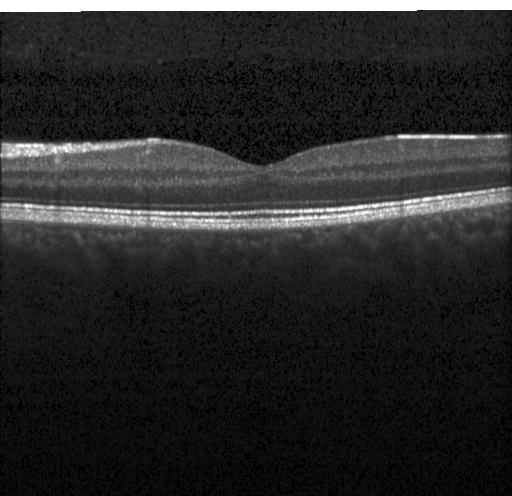
Through the macula · retinal OCT cross-section · Heidelberg Spectralis — Finding: neither choroidal neovascularization, diabetic macular edema, nor drusen.